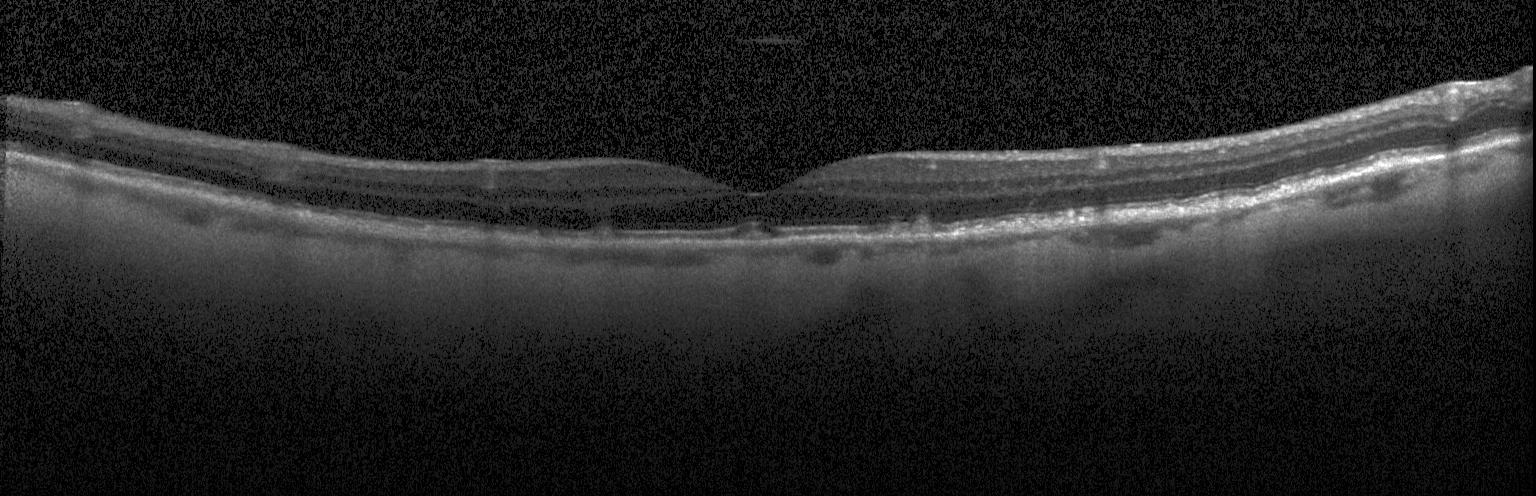

SD-OCT; instrument: Heidelberg Spectralis; optical coherence tomography scan
Impression: multiple drusen.